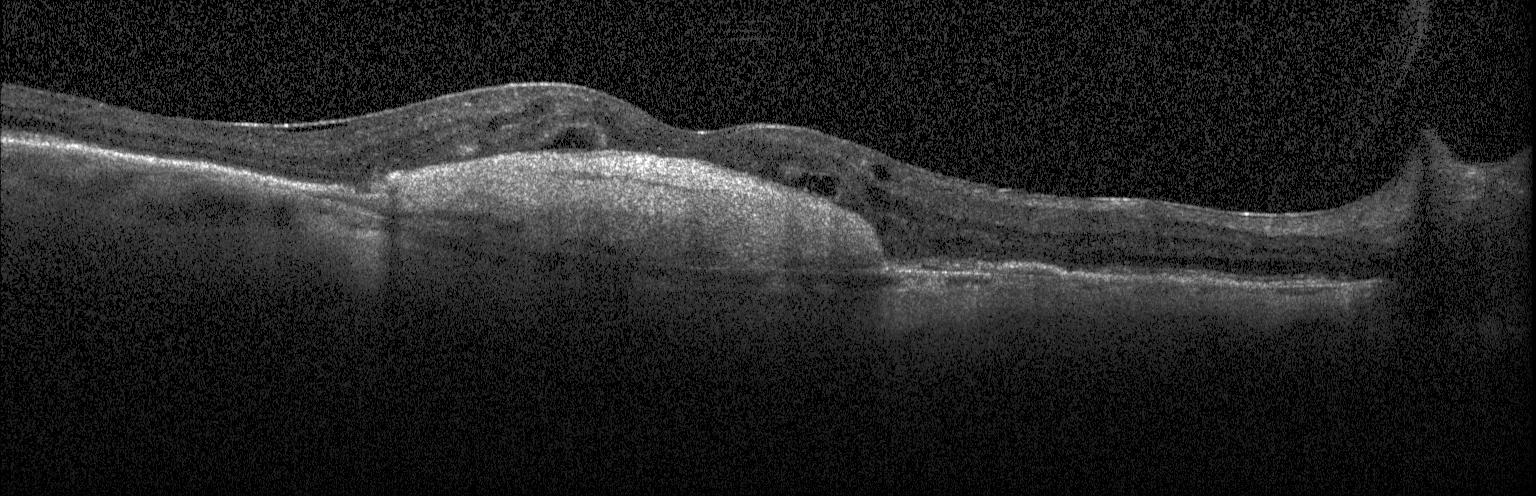

Acquired on a Heidelberg Spectralis; retinal OCT cross-section.
Impression: choroidal neovascularization (CNV).